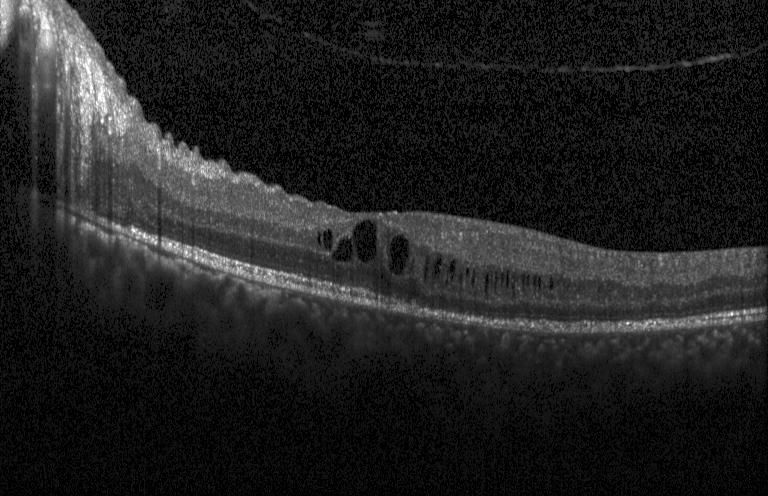 OCT line scan — Macular OCT: diabetic macular edema.